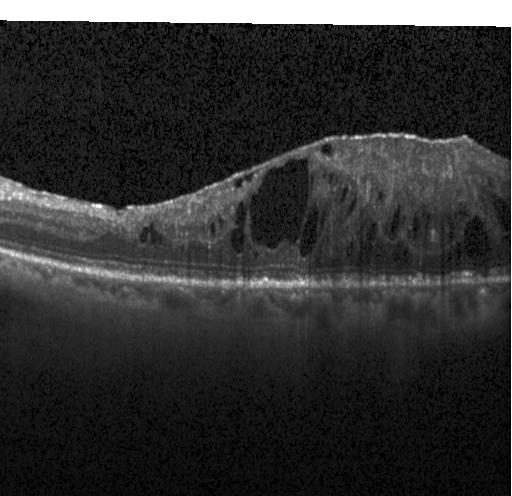

Optical coherence tomography scan — Assessment: diabetic macular edema.